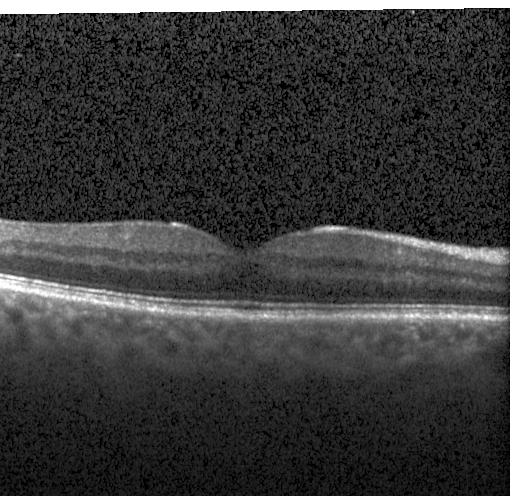
OCT B-scan. Finding: no choroidal neovascularization, diabetic macular edema, or drusen.